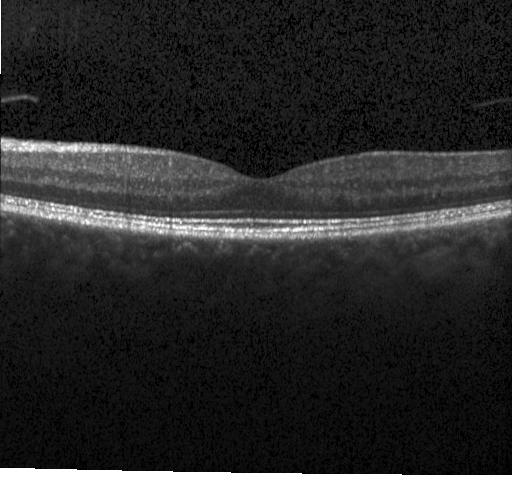

No CNV, no DME, and no drusen.